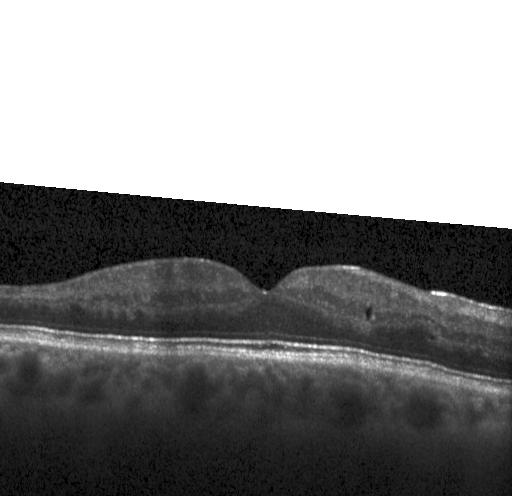
OCT line scan
Assessment: diabetic macular edema.